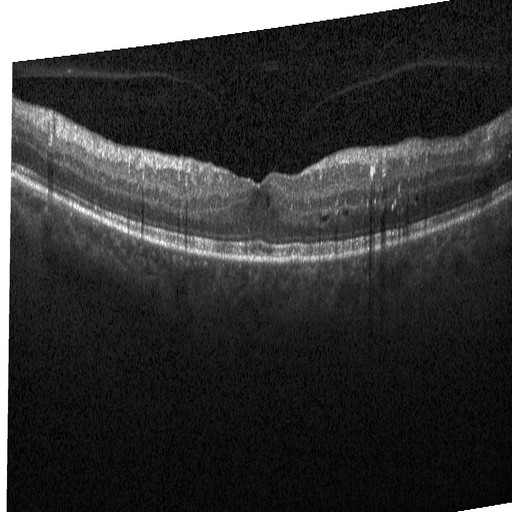

Diabetic macular edema.